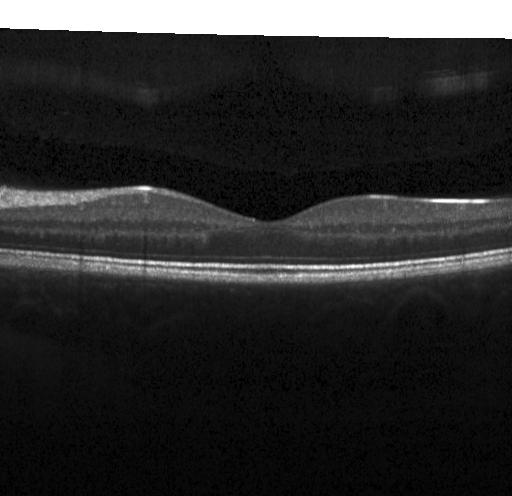
Optical coherence tomography scan — No choroidal neovascularization, no diabetic macular edema, and no drusen.